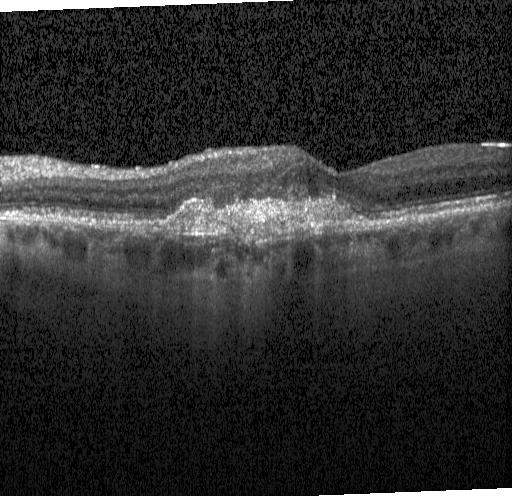 Spectral-domain OCT B-scan: choroidal neovascularization.